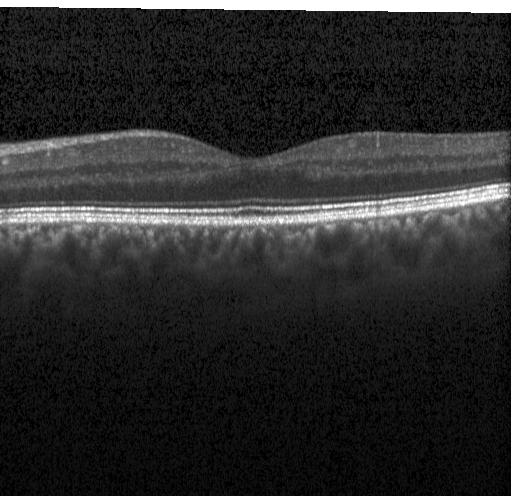

Horizontal scan through the fovea; instrument: Heidelberg Spectralis; optical coherence tomography B-scan; spectral-domain OCT — No evidence of choroidal neovascularization, diabetic macular edema, or drusen.